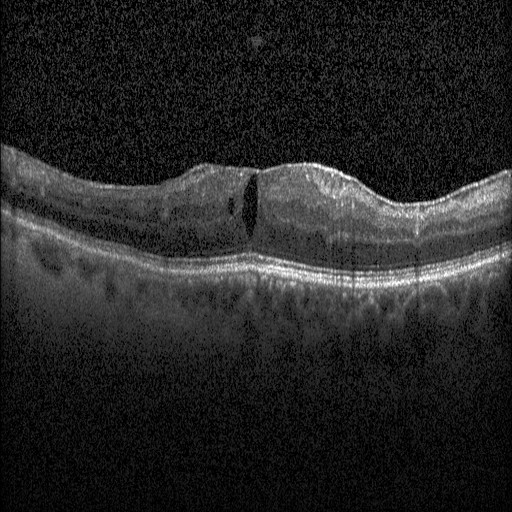

Spectral-domain OCT. Macular scan. OCT line scan
Finding: diabetic macular edema (DME).